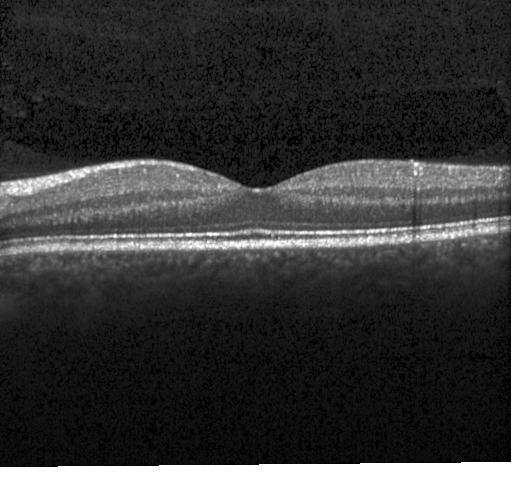

Dx: neither choroidal neovascularization, diabetic macular edema, nor drusen.